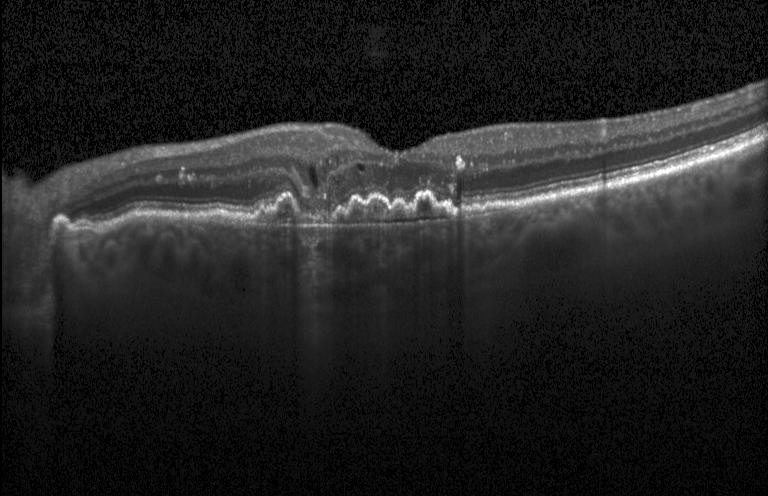
SD-OCT. Instrument: Heidelberg Spectralis. Retinal OCT B-scan. Macular scan
The scan shows a choroidal neovascular membrane.